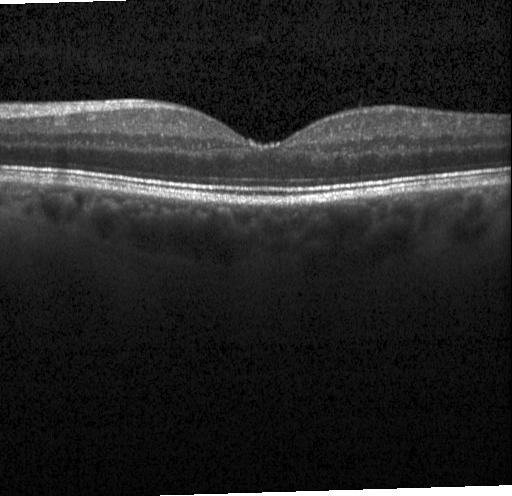

Impression: no choroidal neovascularization, no diabetic macular edema, and no drusen.